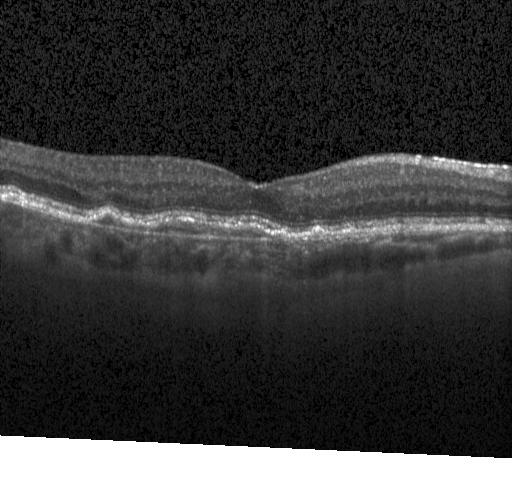
Spectral-domain OCT; OCT B-scan.
Diagnosis: choroidal neovascularization.